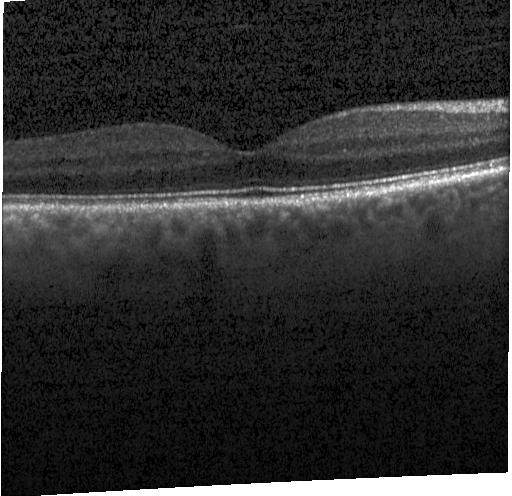

Heidelberg Spectralis; optical coherence tomography scan. Diagnosis: neither CNV, DME, nor drusen.